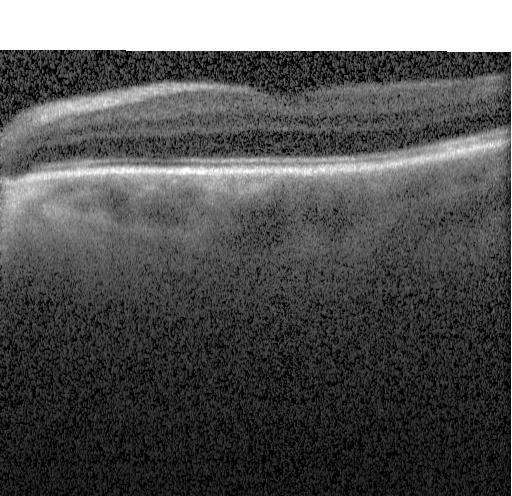 Macular OCT: no CNV, DME, or drusen.